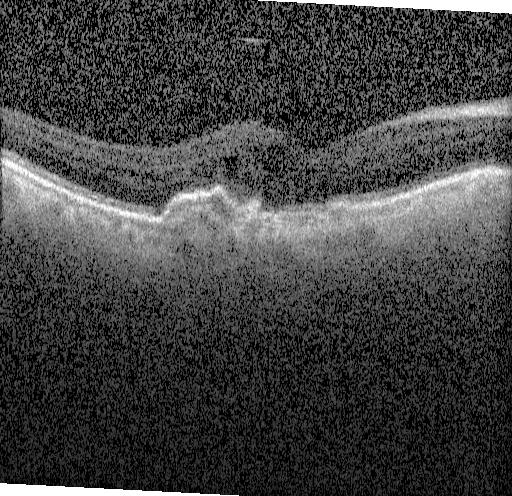
Centered on the fovea, OCT B-scan.
Macular OCT: CNV.